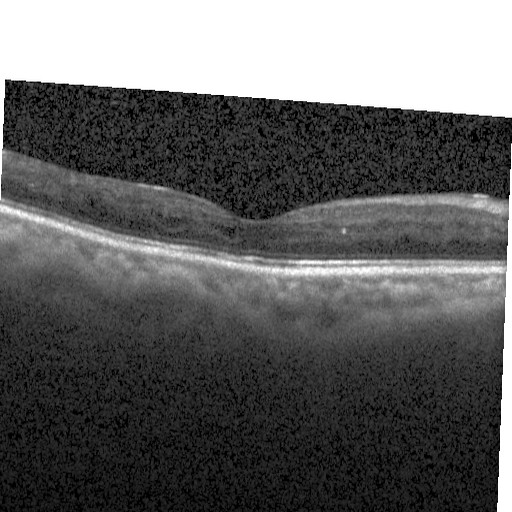

Retinal OCT cross-section.
Impression: DME.